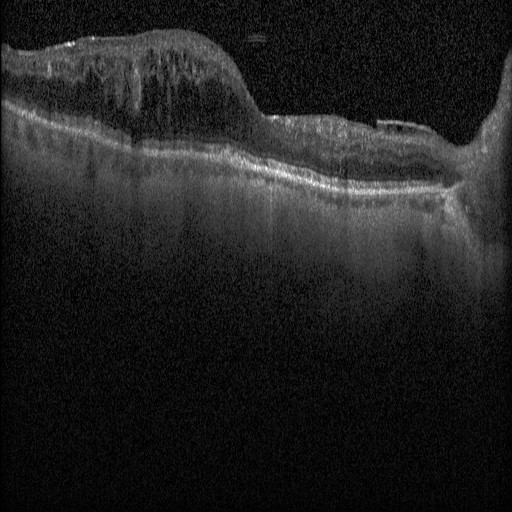 Spectral-domain OCT B-scan: diabetic macular edema.